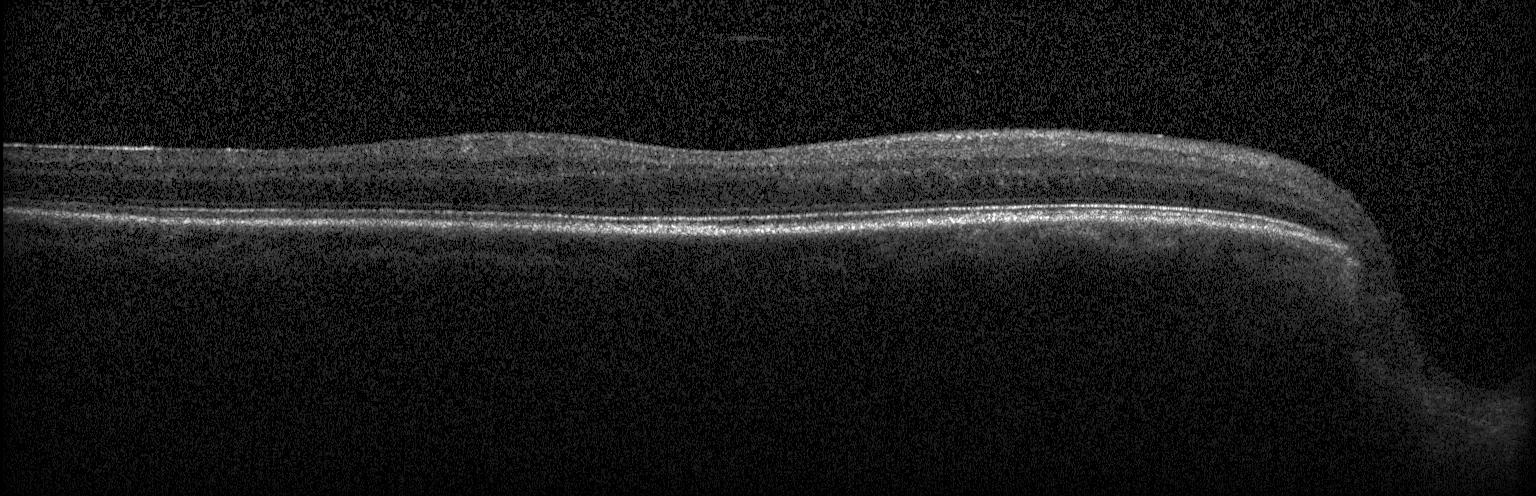

Retinal OCT cross-section.
This B-scan demonstrates no evidence of choroidal neovascularization, diabetic macular edema, or drusen.